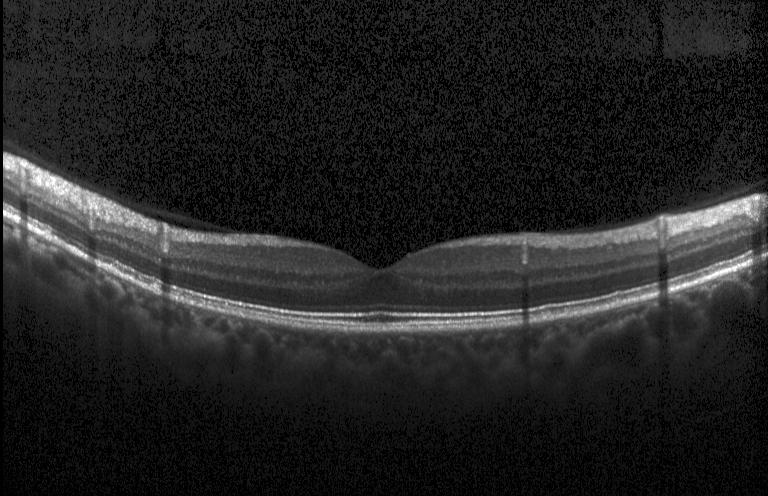 OCT B-scan, instrument: Heidelberg Spectralis, horizontal scan through the fovea
Impression: neither CNV, DME, nor drusen.